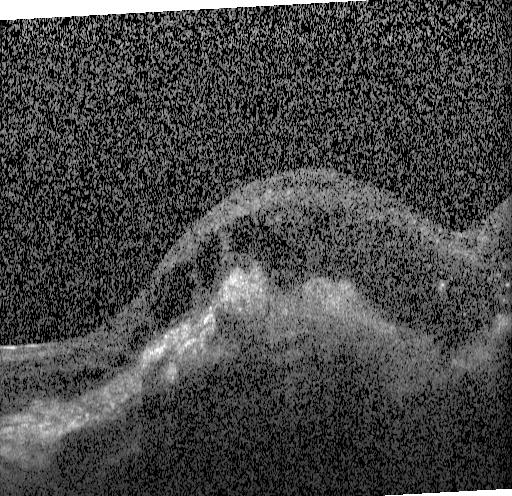
CNV.